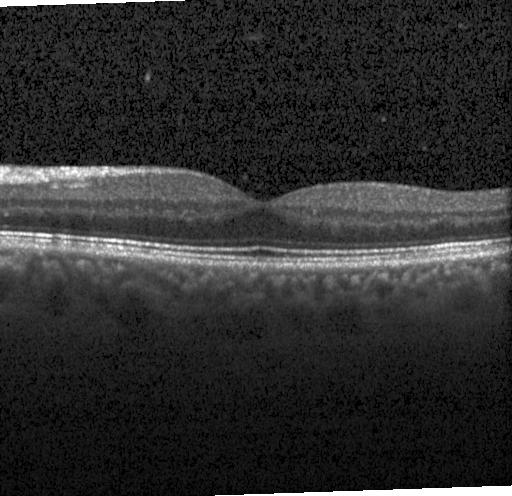
Dx: no evidence of choroidal neovascularization, diabetic macular edema, or drusen.